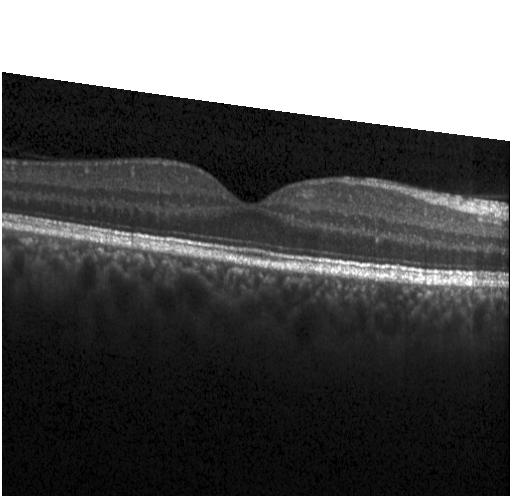
The scan shows neither choroidal neovascularization, diabetic macular edema, nor drusen.